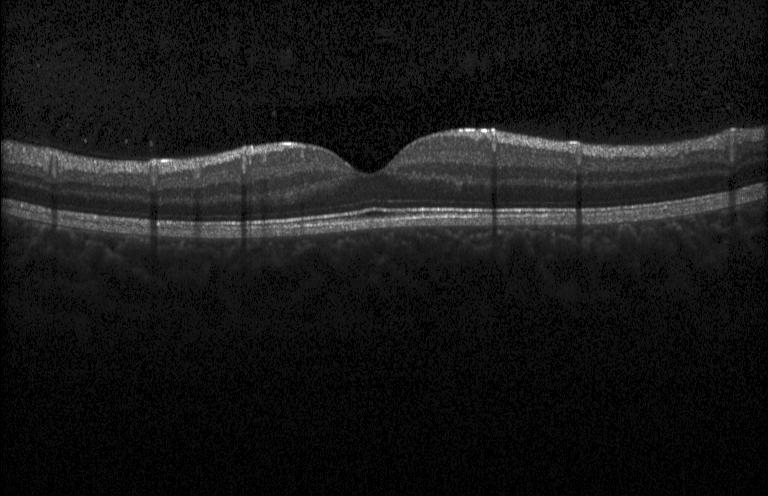
OCT scan showing no choroidal neovascularization, no diabetic macular edema, and no drusen.